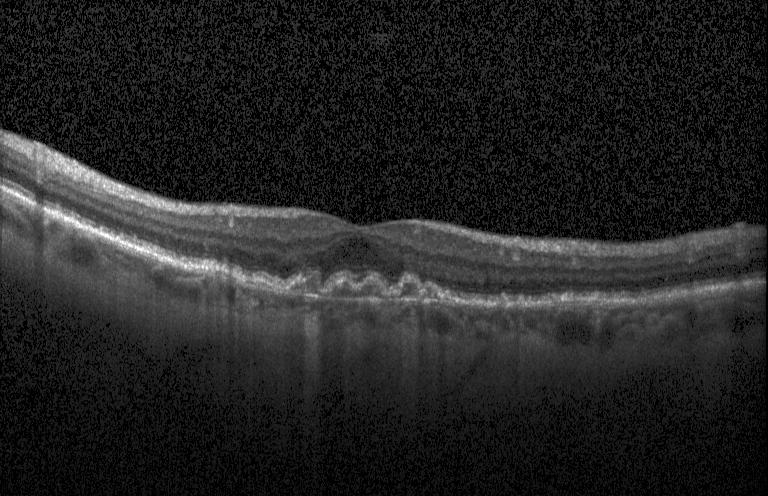

Finding: a choroidal neovascular membrane.